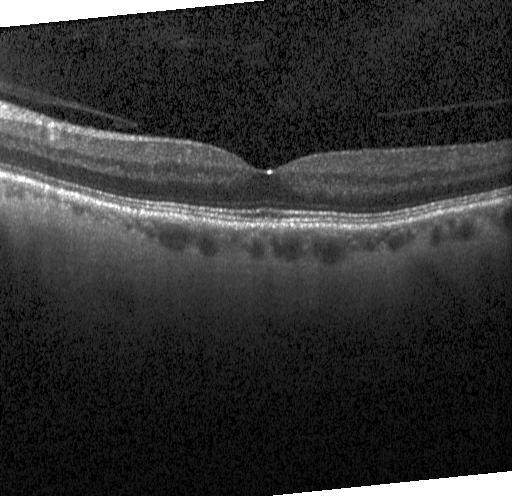 Diagnosis: no choroidal neovascularization, diabetic macular edema, or drusen.